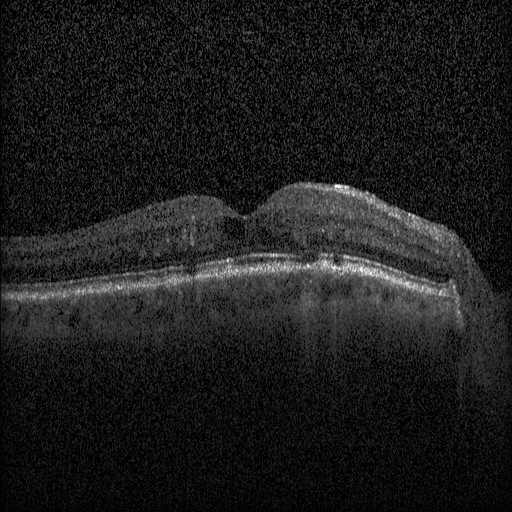 Heidelberg Spectralis OCT system. Macular scan. Optical coherence tomography scan. The scan shows diabetic macular edema (DME).